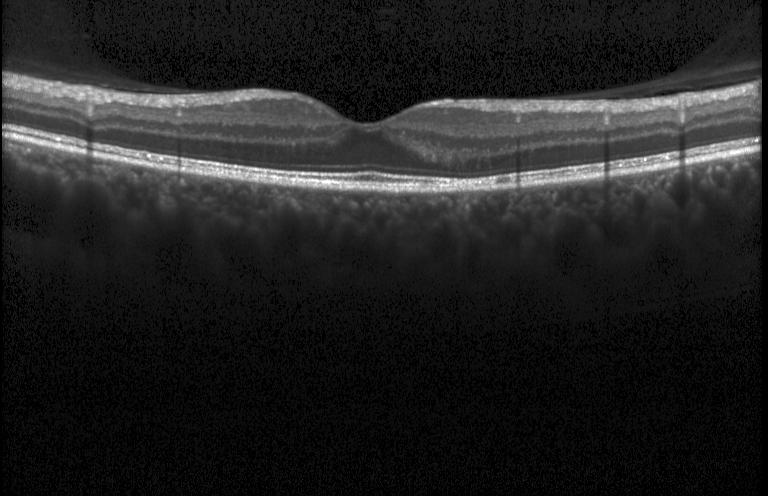
Impression: neither choroidal neovascularization, diabetic macular edema, nor drusen.